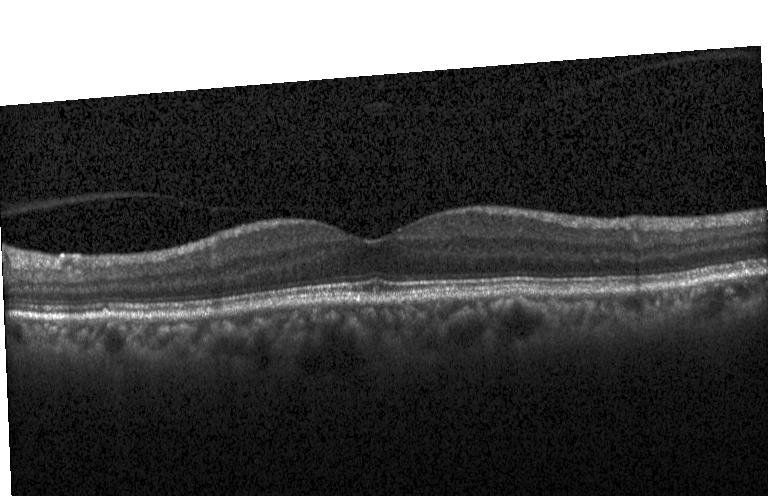

Macular scan; optical coherence tomography scan; Heidelberg Spectralis OCT system; spectral-domain optical coherence tomography.
Finding: no choroidal neovascularization, diabetic macular edema, or drusen.